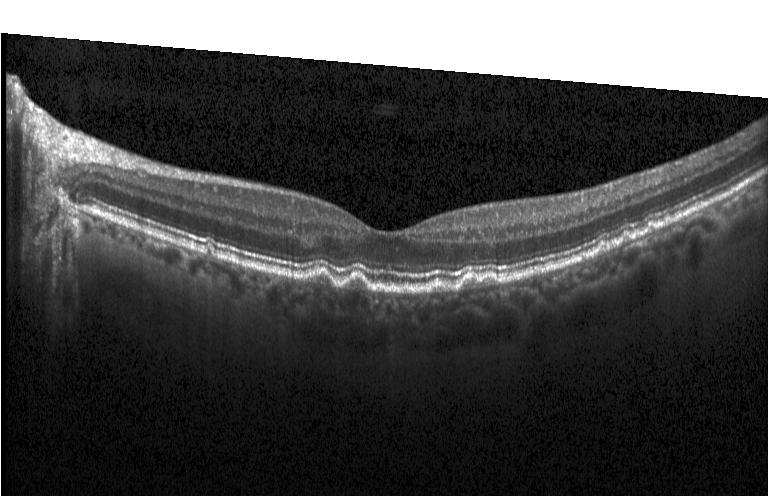 SD-OCT. Centered on the fovea. Heidelberg Spectralis OCT system. Optical coherence tomography B-scan
Dx: drusen.